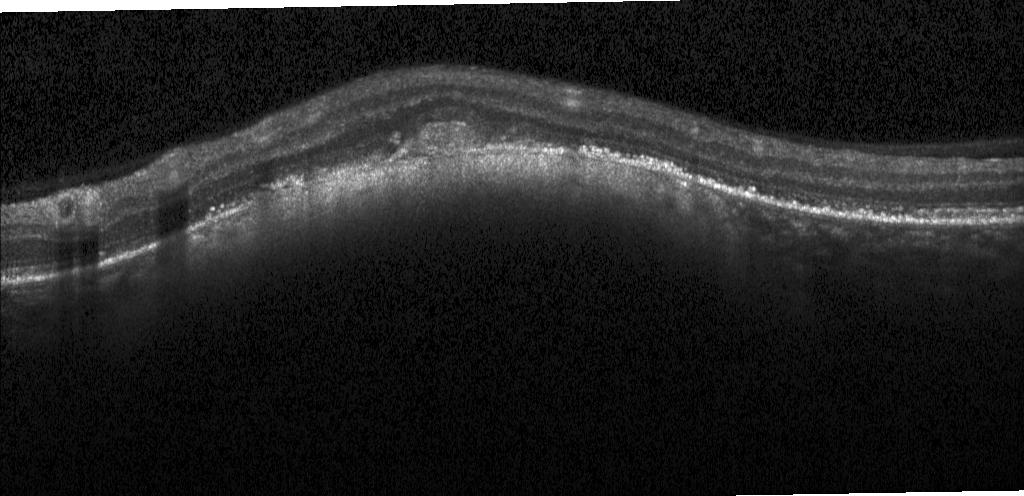
Retinal OCT B-scan, spectral-domain optical coherence tomography. Finding: choroidal neovascularization.